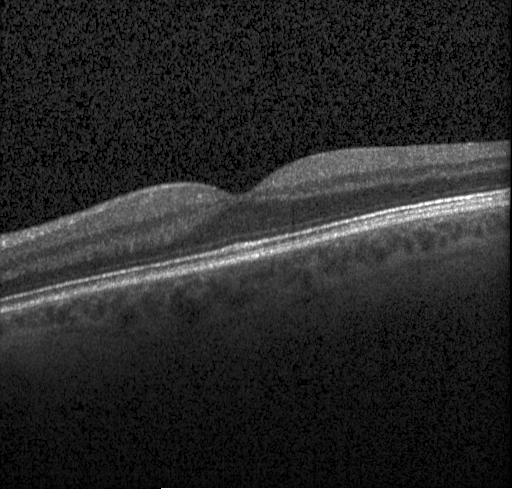 Spectral-domain OCT, optical coherence tomography B-scan, instrument: Heidelberg Spectralis
This B-scan demonstrates no CNV, DME, or drusen.